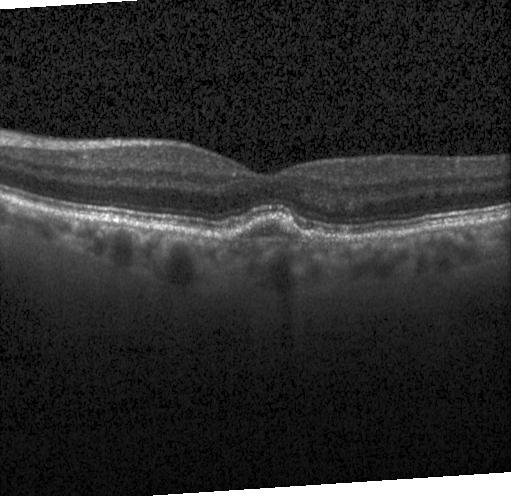

Retinal OCT cross-section — OCT finding: a choroidal neovascular membrane.